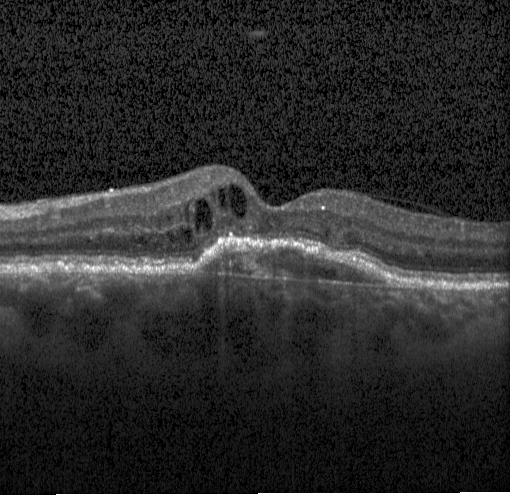
Centered on the fovea; OCT line scan
The scan shows CNV.